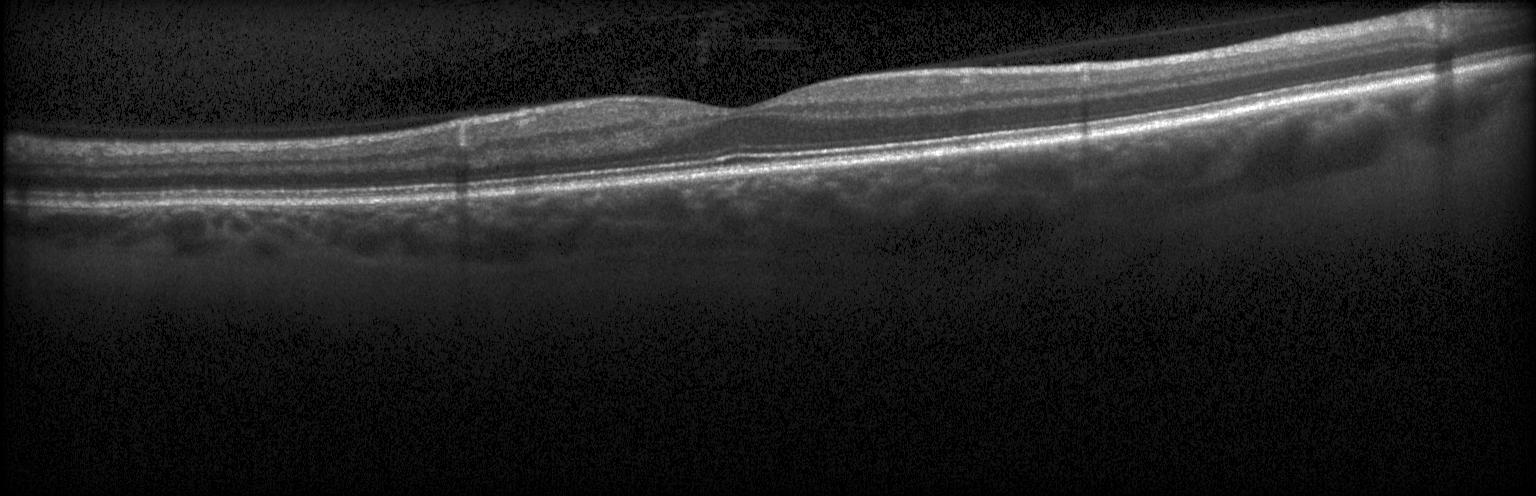
SD-OCT, Heidelberg Spectralis OCT system, retinal OCT B-scan. The scan shows no evidence of CNV, DME, or drusen.